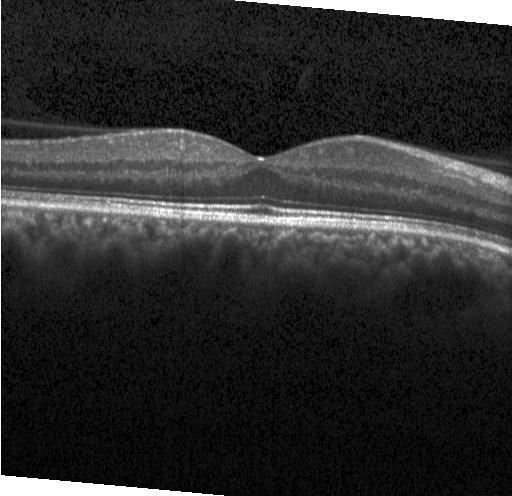

Macular OCT: neither choroidal neovascularization, diabetic macular edema, nor drusen.